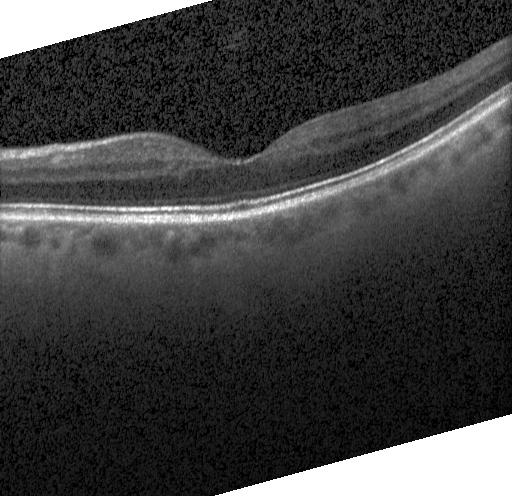 Acquired on a Heidelberg Spectralis; OCT line scan
Dx: no choroidal neovascularization, no diabetic macular edema, and no drusen.